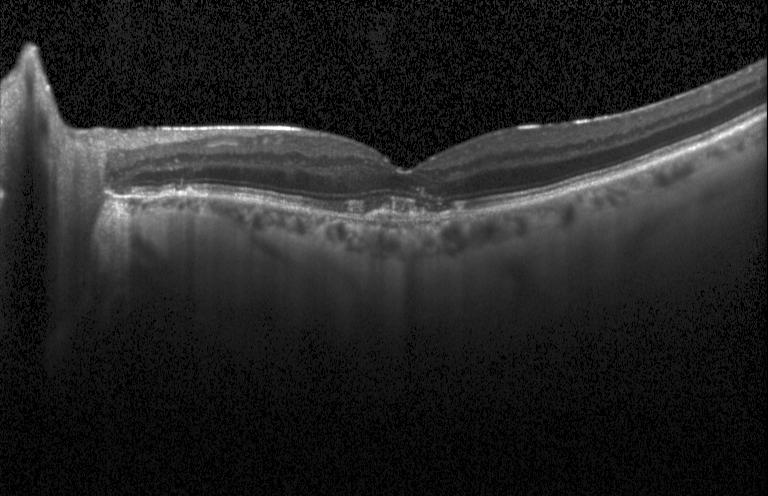

Horizontal scan through the fovea · retinal OCT B-scan. Dx: a choroidal neovascular membrane.